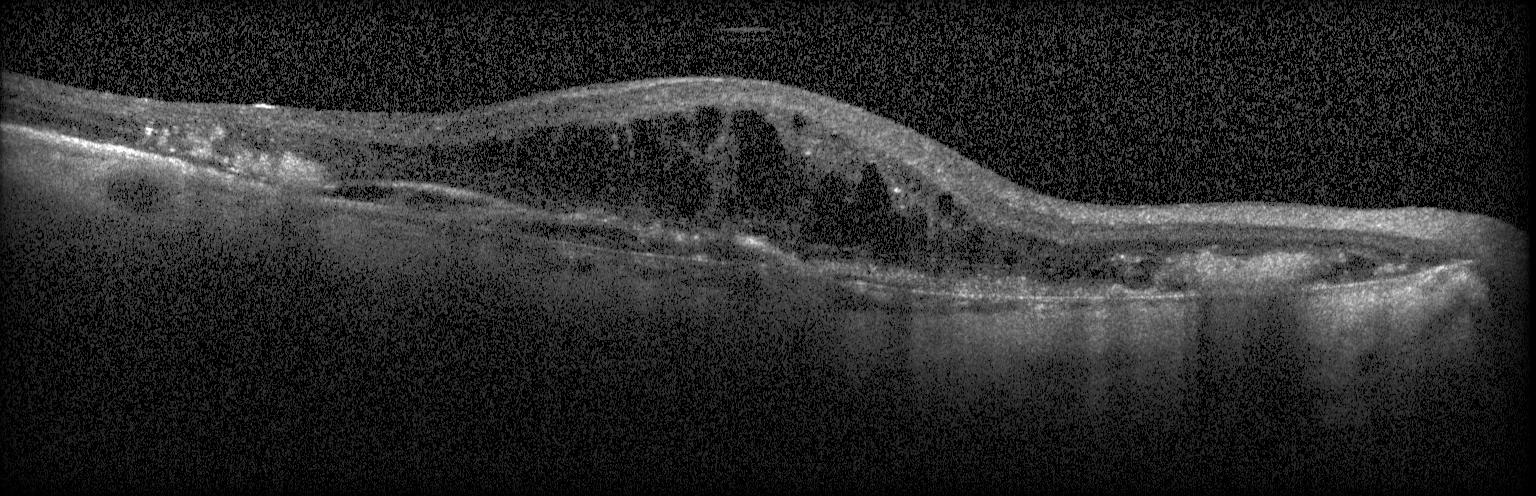
Retinal OCT B-scan — Macular OCT: choroidal neovascularization (CNV).